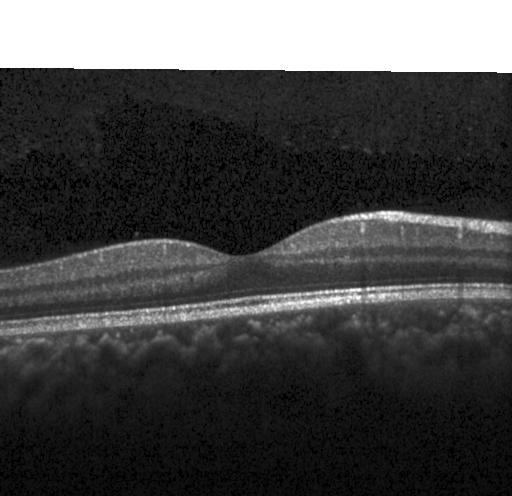
Retinal OCT B-scan
OCT finding: no choroidal neovascularization, diabetic macular edema, or drusen.